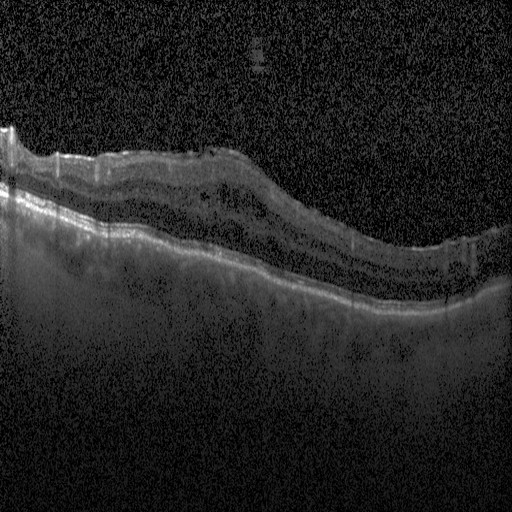

Heidelberg Spectralis OCT system, centered on the fovea, optical coherence tomography scan. Impression: DME.